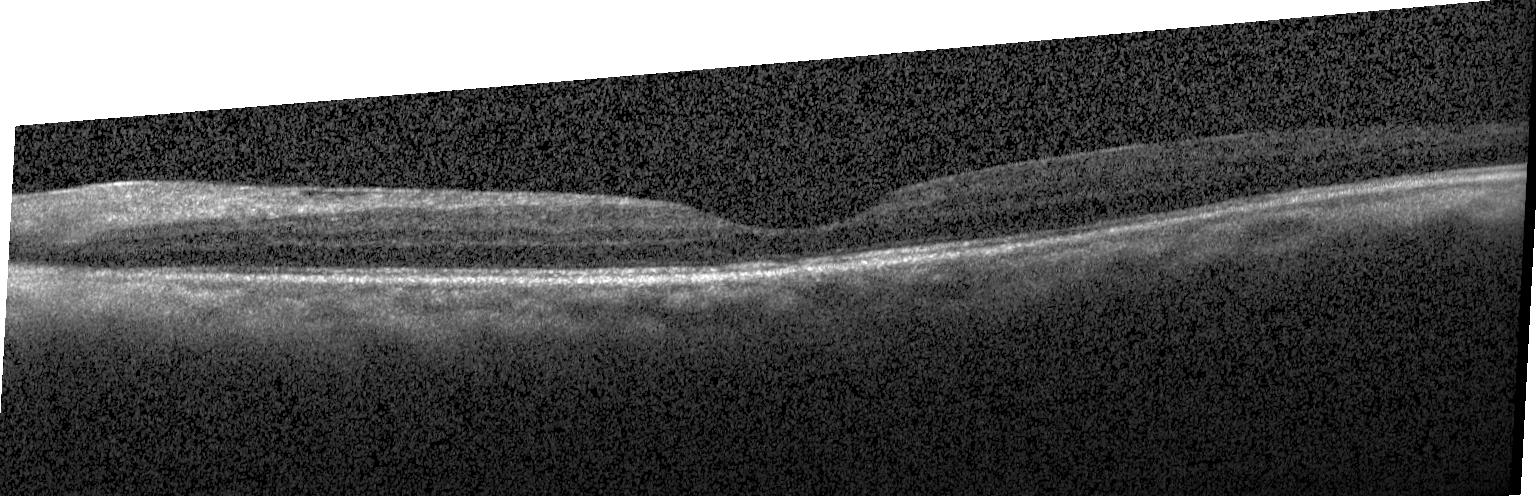 Macular scan, SD-OCT, retinal OCT cross-section, instrument: Heidelberg Spectralis — OCT finding: no evidence of choroidal neovascularization, diabetic macular edema, or drusen.